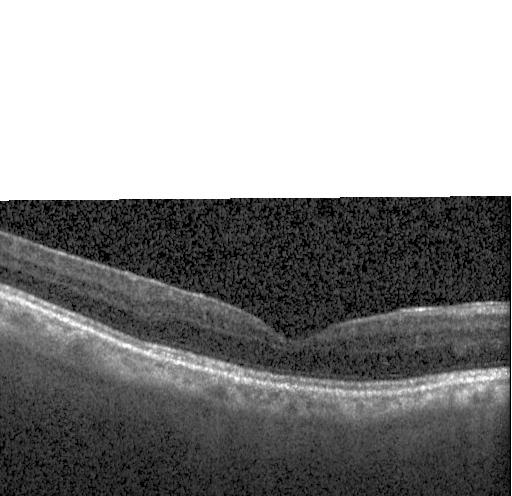
Acquired on a Heidelberg Spectralis, retinal OCT B-scan. Impression: neither CNV, DME, nor drusen.